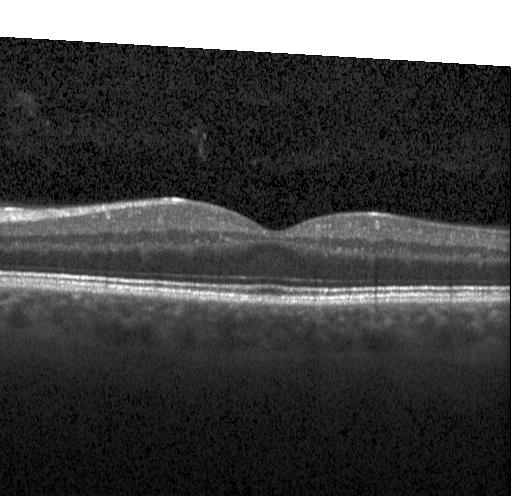
Horizontal scan through the fovea. OCT B-scan. OCT finding: no evidence of CNV, DME, or drusen.